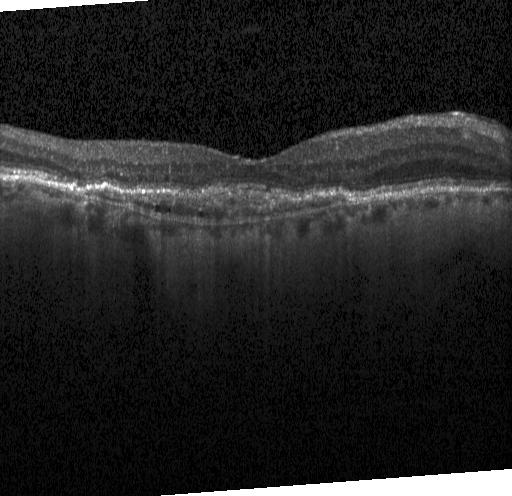
This B-scan demonstrates choroidal neovascularization (CNV).